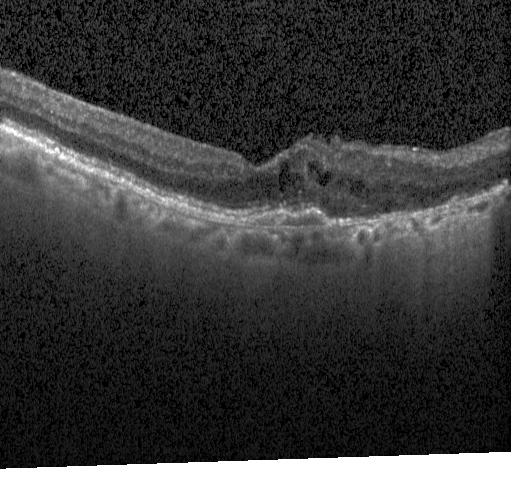
Macular scan; optical coherence tomography B-scan
Finding: CNV.